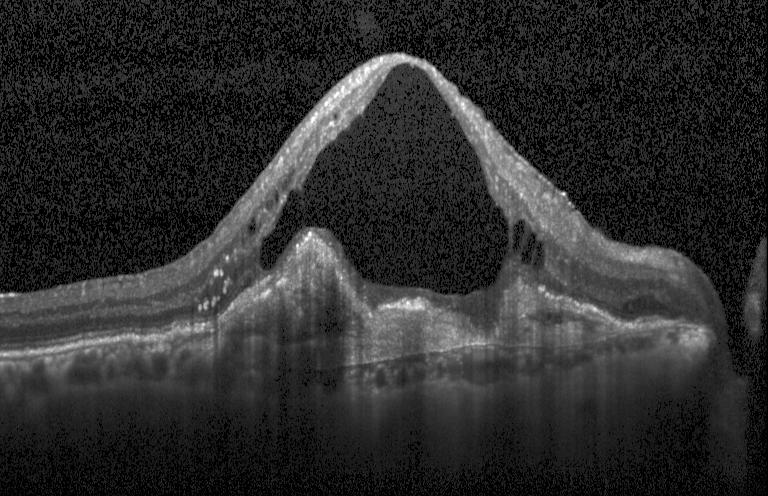

Retinal OCT cross-section.
Finding: choroidal neovascularization (CNV).